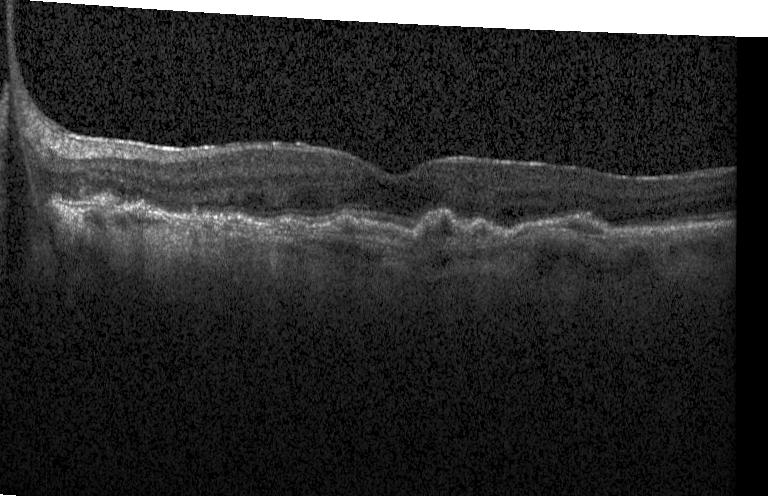
Retinal OCT B-scan. Heidelberg Spectralis. Fovea-centered
Impression: choroidal neovascularization.